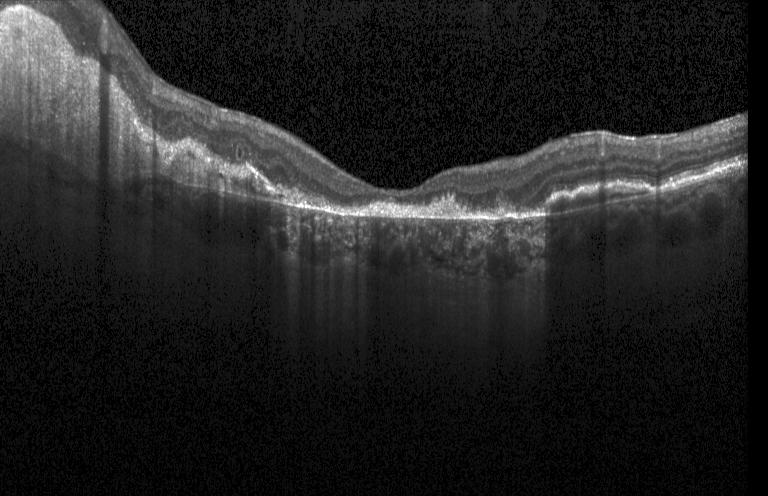 OCT line scan — Finding: choroidal neovascularization (CNV).